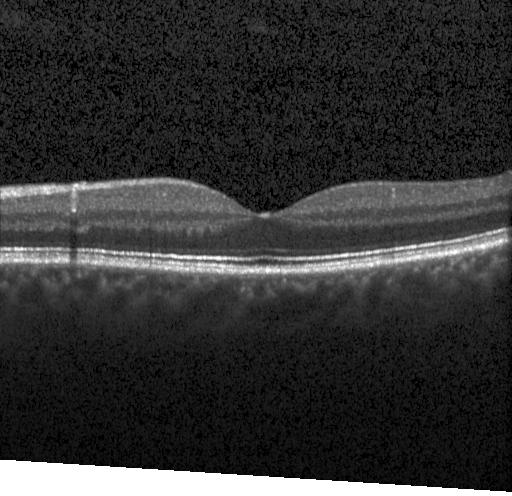 Heidelberg Spectralis OCT system · spectral-domain optical coherence tomography · optical coherence tomography scan · horizontal scan through the fovea. This B-scan demonstrates no CNV, DME, or drusen.